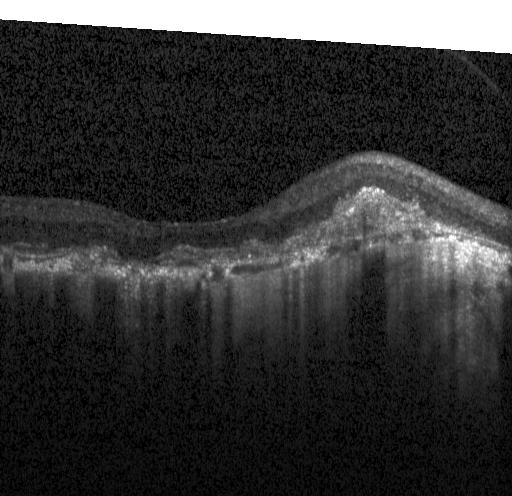 Retinal OCT cross-section — Impression: choroidal neovascularization.